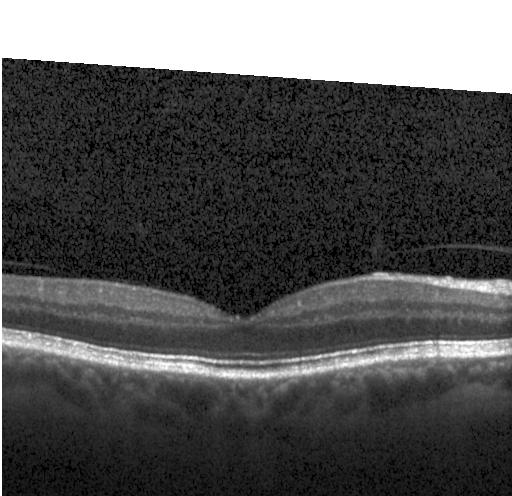 Finding: no choroidal neovascularization, diabetic macular edema, or drusen.